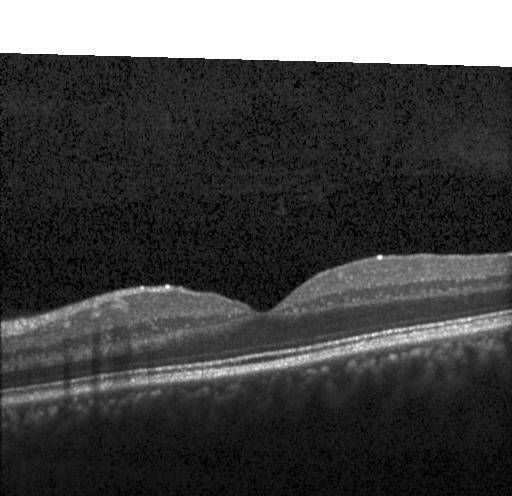

Optical coherence tomography B-scan.
OCT finding: no evidence of choroidal neovascularization, diabetic macular edema, or drusen.